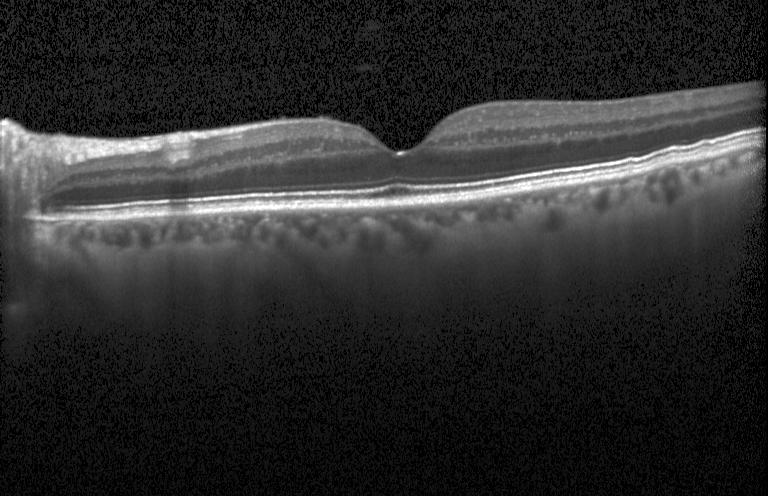 SD-OCT · through the macula · retinal OCT B-scan.
Finding: no choroidal neovascularization, diabetic macular edema, or drusen.